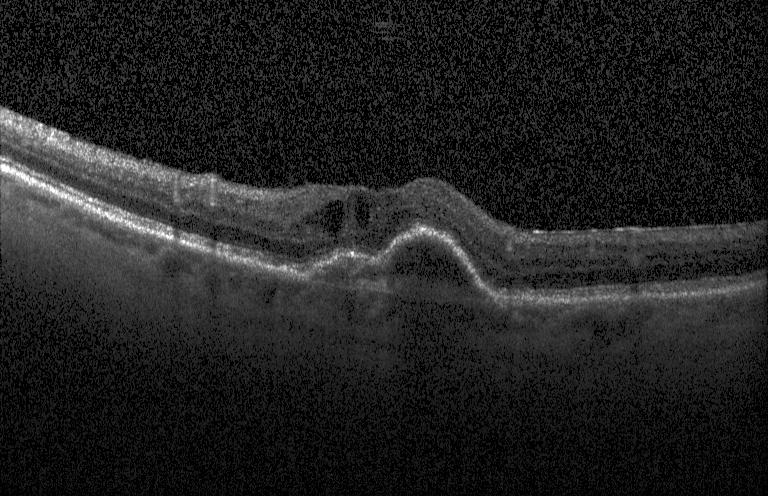 Finding: a choroidal neovascular membrane.